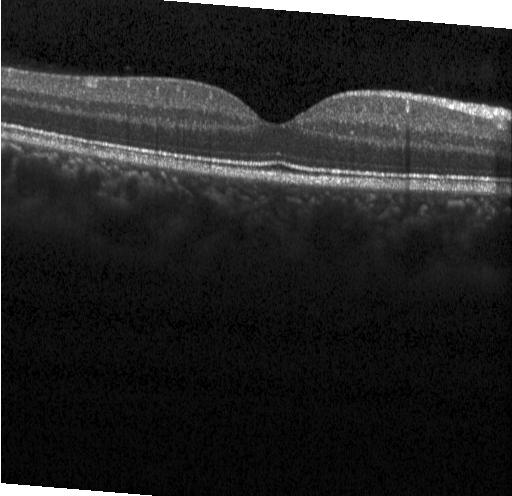 Fovea-centered; optical coherence tomography scan; Heidelberg Spectralis
This B-scan demonstrates no evidence of choroidal neovascularization, diabetic macular edema, or drusen.